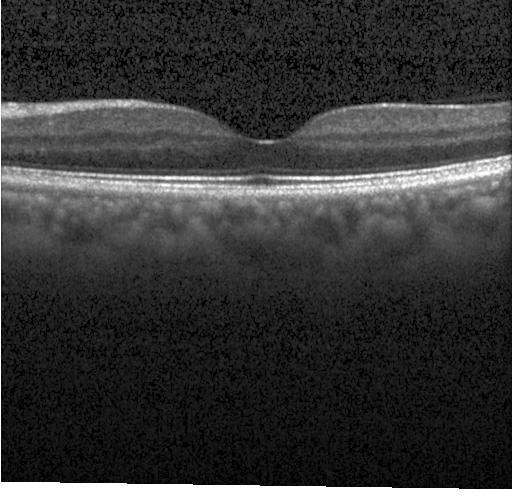

Finding: no choroidal neovascularization, diabetic macular edema, or drusen.